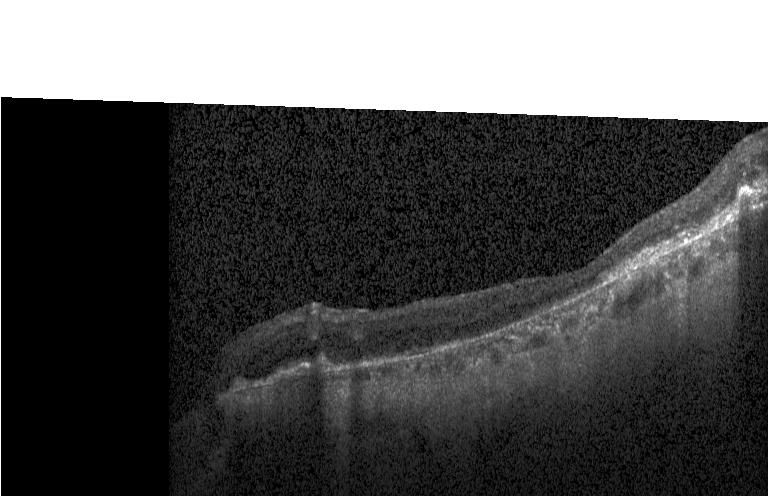 Assessment: a choroidal neovascular membrane.